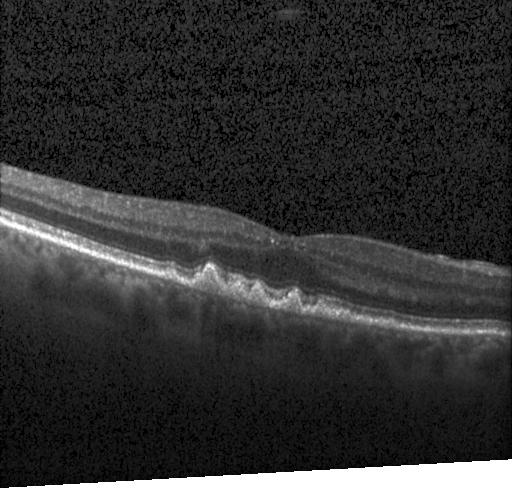 OCT line scan.
Impression: sub-RPE drusenoid deposits.